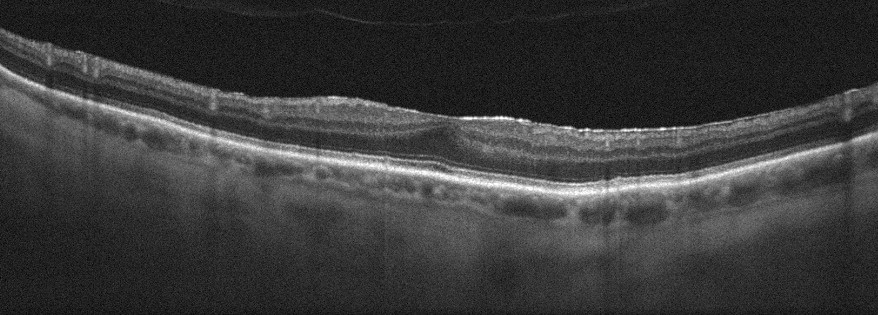

Dx: epiretinal membrane (ERM).